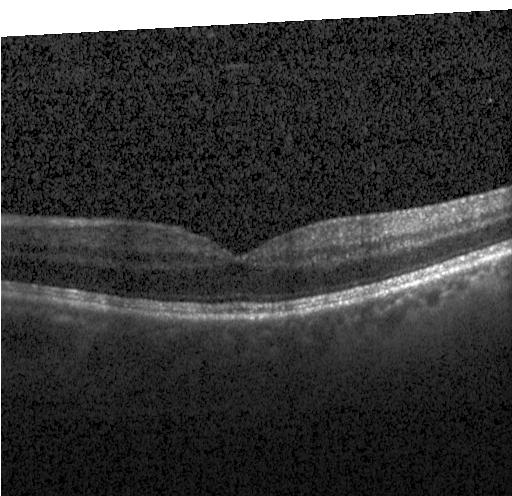

OCT line scan.
Diagnosis: no choroidal neovascularization, no diabetic macular edema, and no drusen.